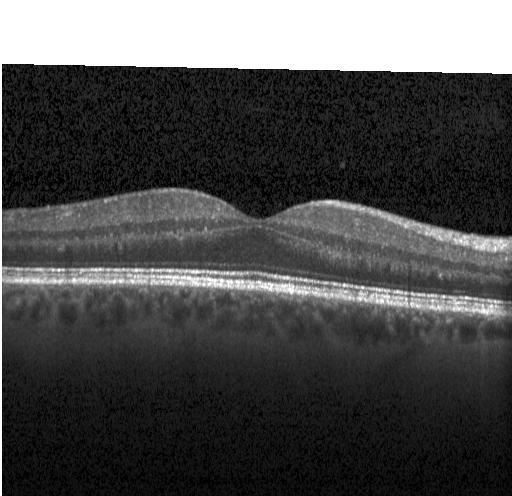 OCT line scan · SD-OCT.
This B-scan demonstrates neither CNV, DME, nor drusen.